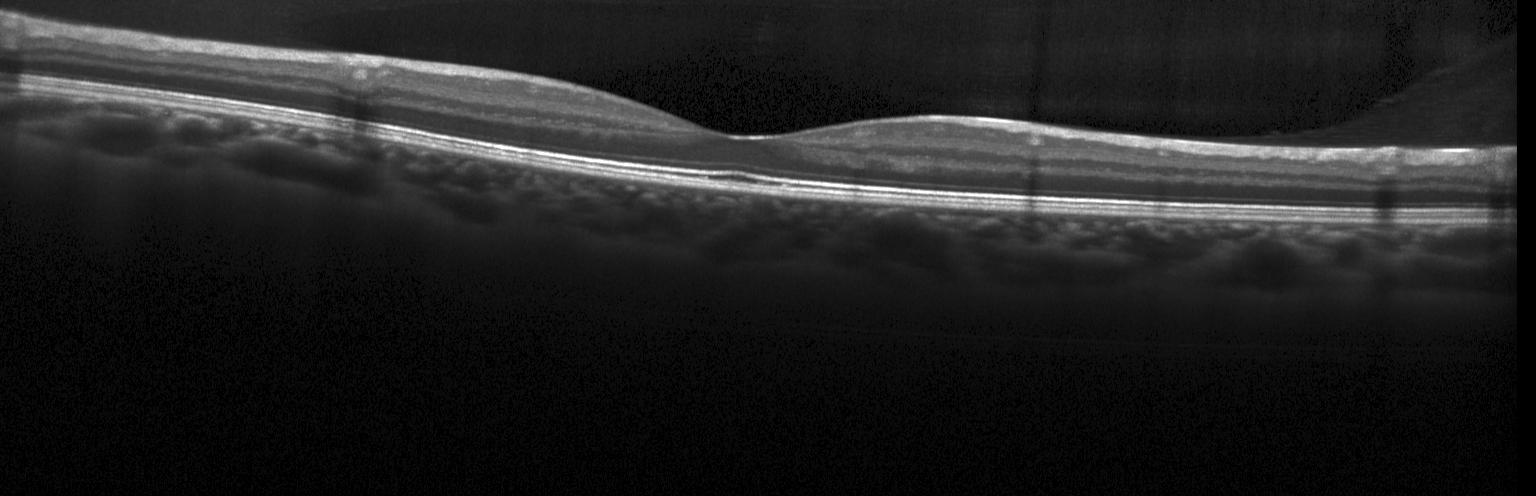

Retinal OCT cross-section showing no choroidal neovascularization, no diabetic macular edema, and no drusen.